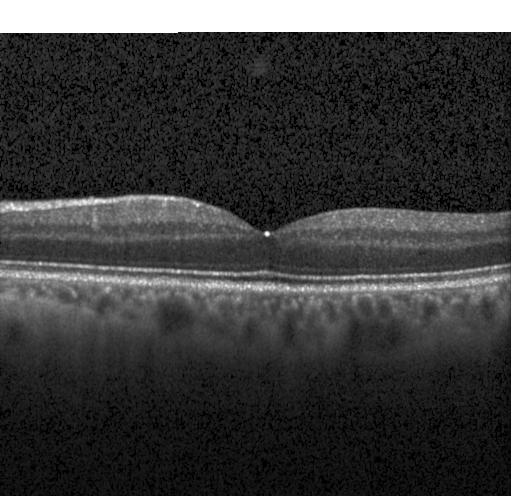

OCT finding: no evidence of choroidal neovascularization, diabetic macular edema, or drusen.